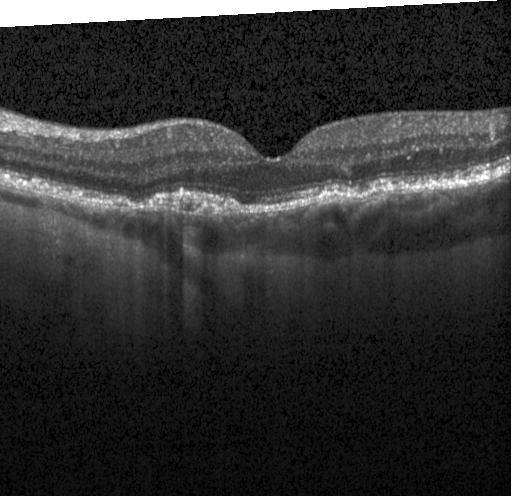 Impression: a choroidal neovascular membrane.